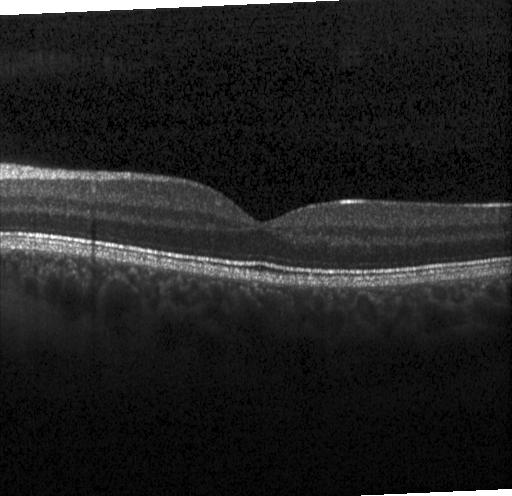

Spectral-domain optical coherence tomography, OCT line scan, Heidelberg Spectralis OCT system, fovea-centered.
Assessment: neither CNV, DME, nor drusen.